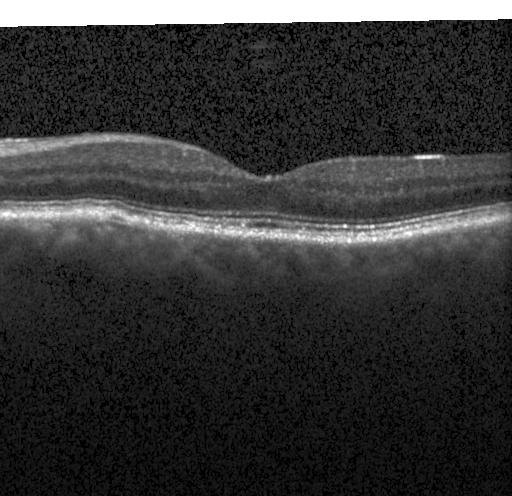 Fovea-centered · spectral-domain optical coherence tomography · instrument: Heidelberg Spectralis · OCT B-scan
OCT finding: multiple drusen.